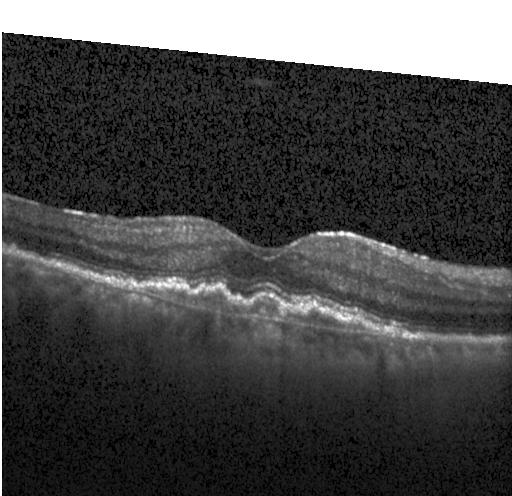 Spectral-domain OCT B-scan: a choroidal neovascular membrane.